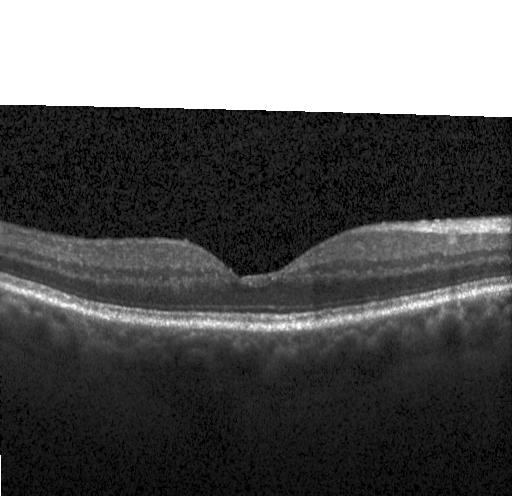

Macular OCT demonstrating no choroidal neovascularization, diabetic macular edema, or drusen.